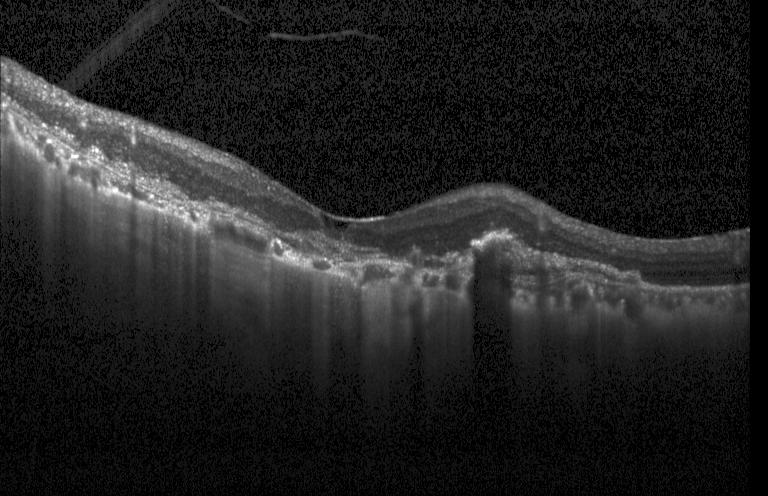
Through the macula. OCT B-scan. Acquired on a Heidelberg Spectralis.
Impression: choroidal neovascularization (CNV).